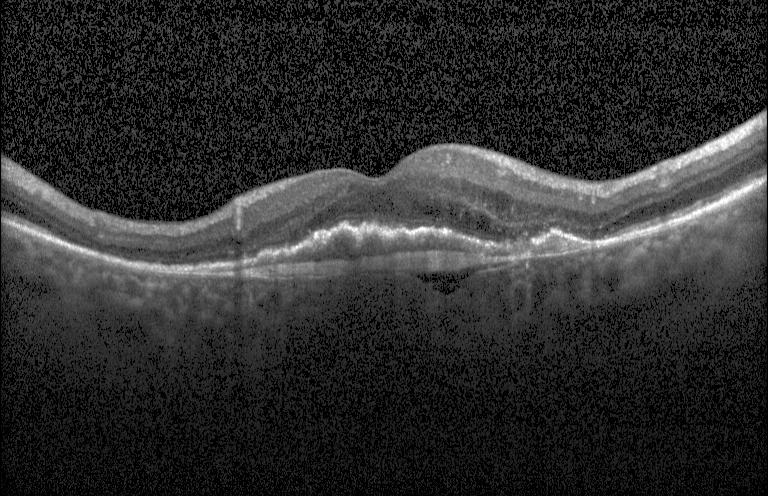

Fovea-centered. Optical coherence tomography B-scan. Spectral-domain optical coherence tomography
OCT finding: a choroidal neovascular membrane.